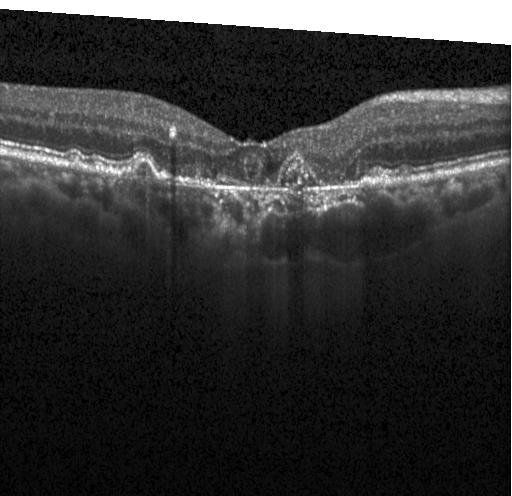

OCT line scan — OCT finding: a choroidal neovascular membrane.